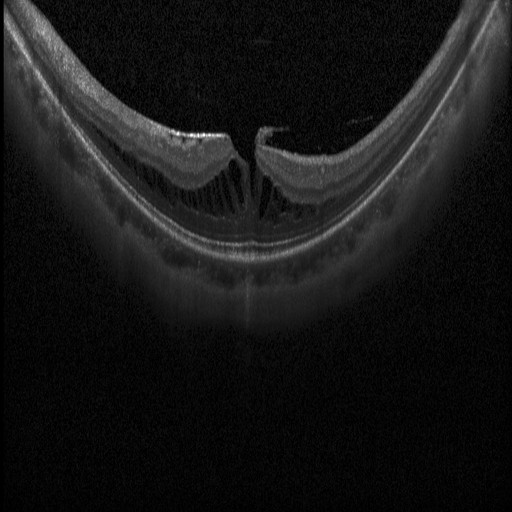
The scan shows diabetic macular edema (DME).